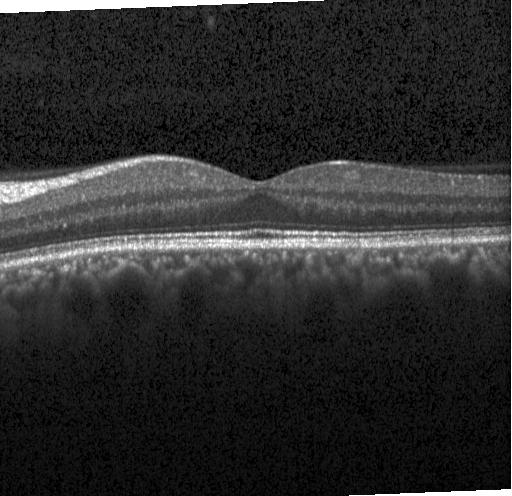

This B-scan demonstrates no CNV, DME, or drusen.